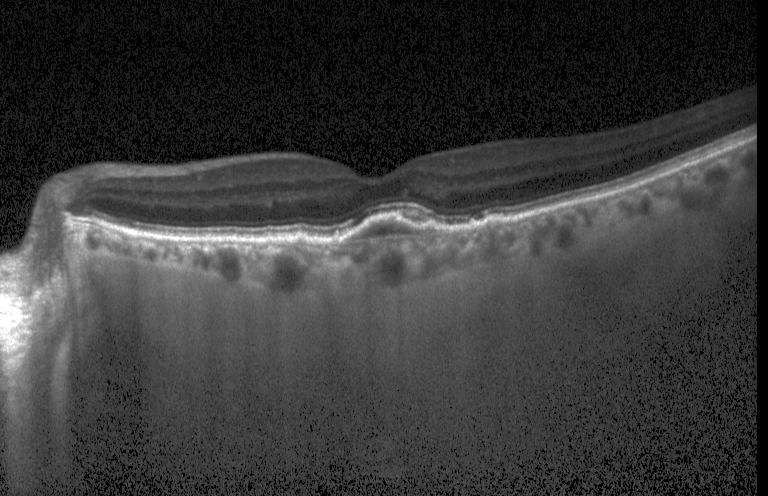
OCT finding: a choroidal neovascular membrane.